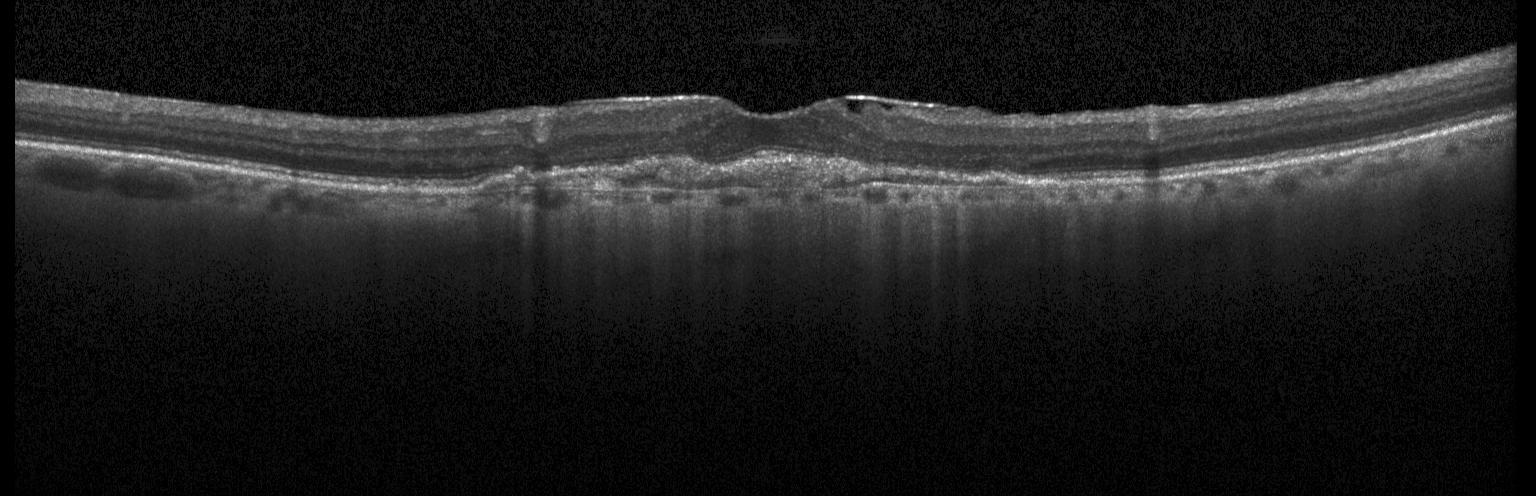

Spectral-domain OCT B-scan: choroidal neovascularization (CNV).